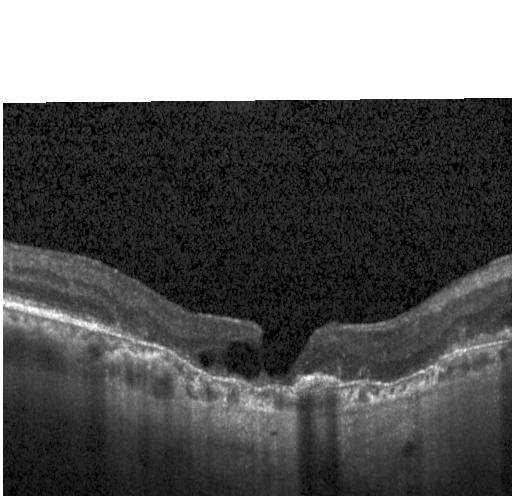 Retinal OCT B-scan — Macular OCT: a choroidal neovascular membrane.